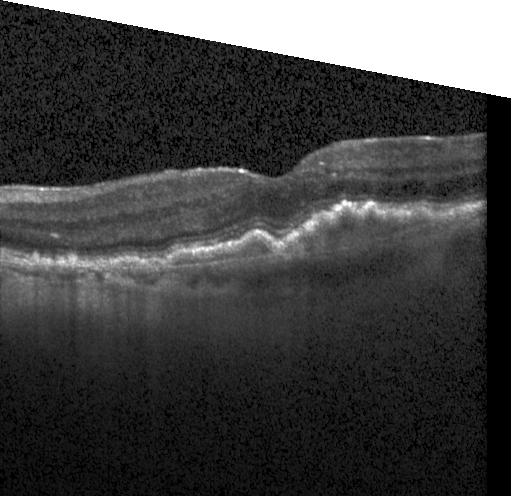 Macular scan. OCT line scan. Heidelberg Spectralis
Impression: a choroidal neovascular membrane.